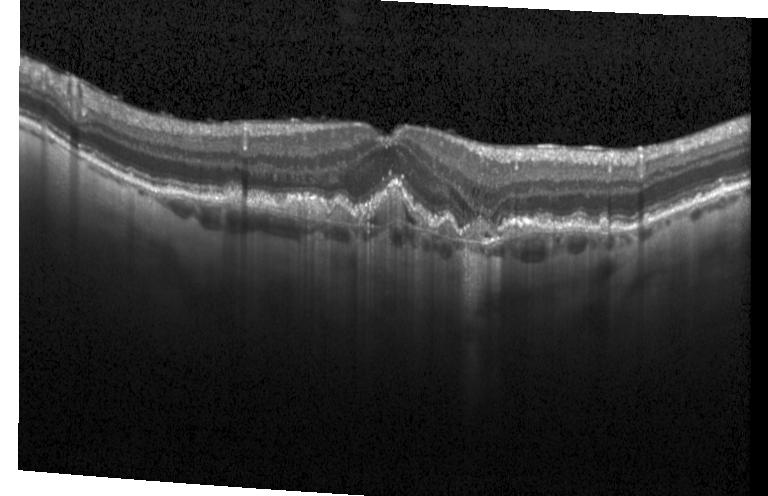
OCT B-scan showing a choroidal neovascular membrane.